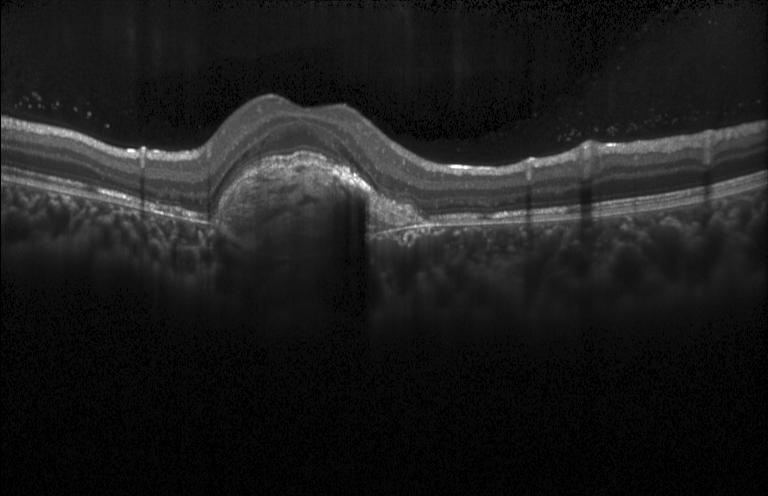

This B-scan demonstrates choroidal neovascularization.